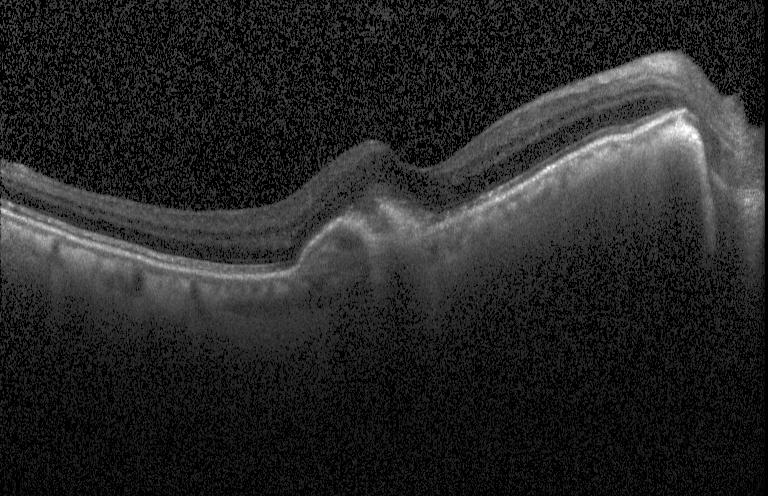
Heidelberg Spectralis OCT system. Retinal OCT B-scan. Centered on the fovea
Dx: a choroidal neovascular membrane.